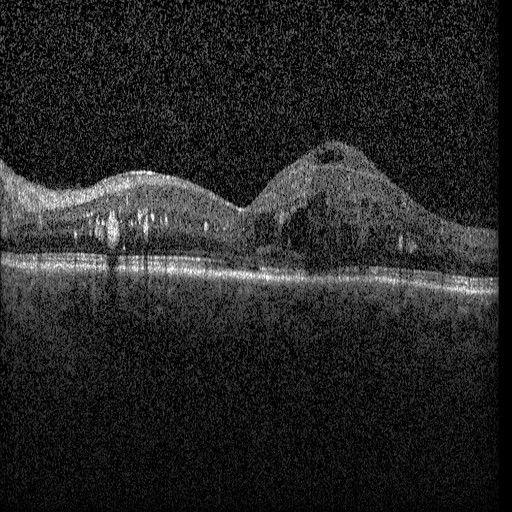

Optical coherence tomography B-scan, through the macula
Dx: diabetic macular edema (DME).